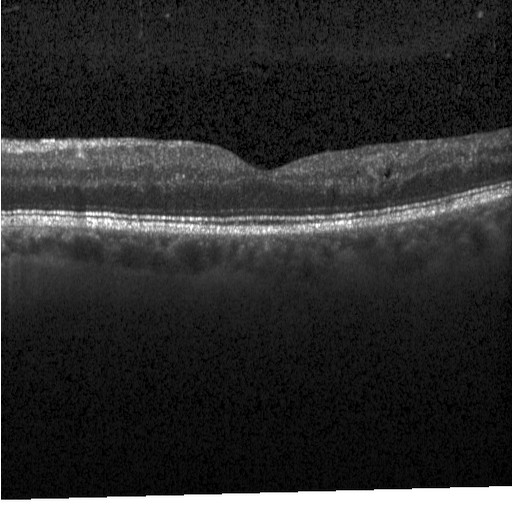
OCT line scan.
Assessment: diabetic macular edema (DME).